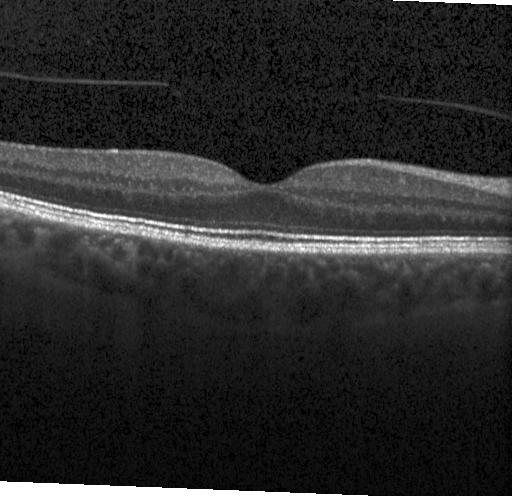

Impression: no CNV, no DME, and no drusen.